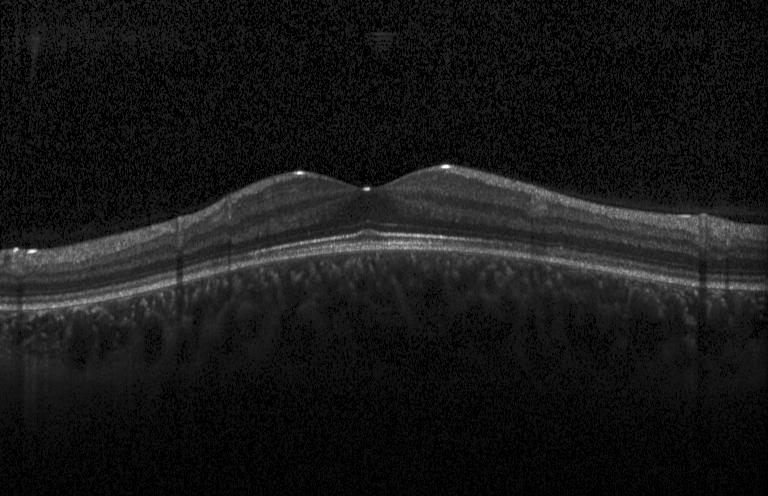

No choroidal neovascularization, diabetic macular edema, or drusen.